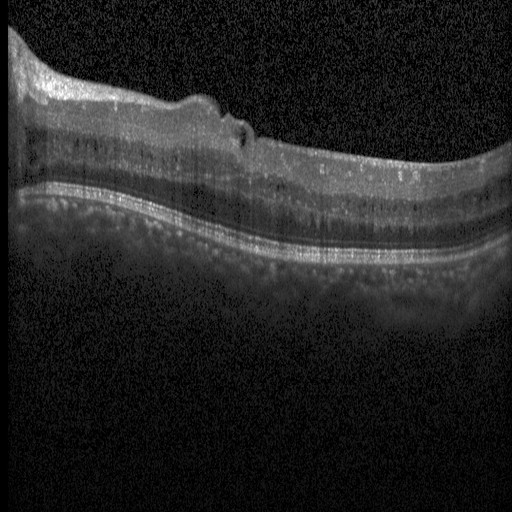 Horizontal scan through the fovea, Heidelberg Spectralis, retinal OCT B-scan. Diagnosis: DME.